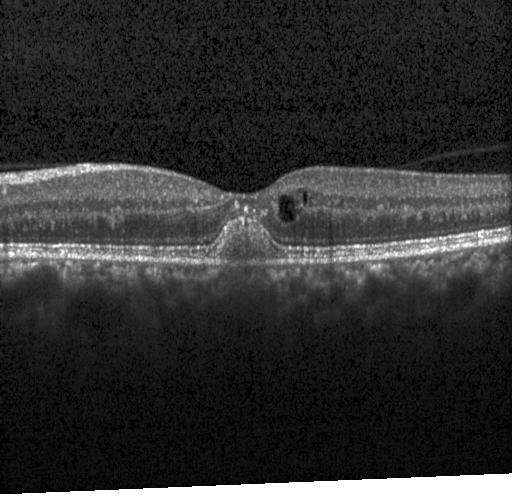 OCT B-scan.
OCT finding: a choroidal neovascular membrane.